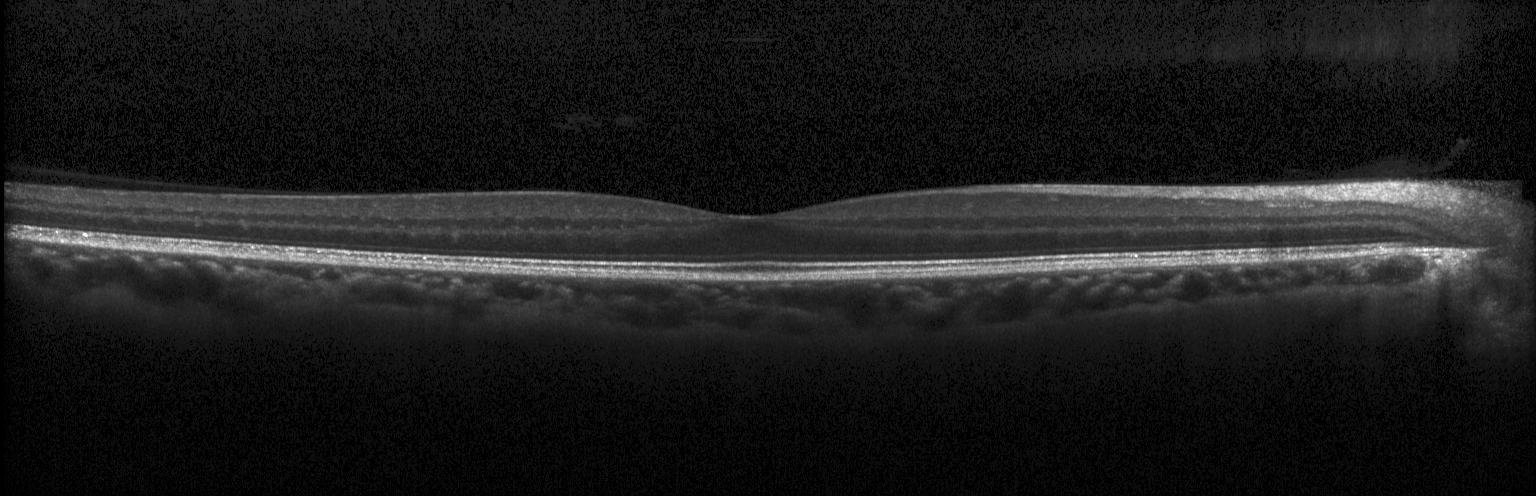
Retinal OCT B-scan. No CNV, DME, or drusen.